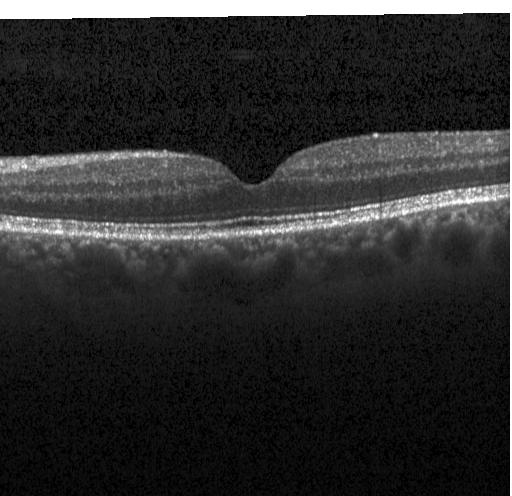
Assessment: no evidence of choroidal neovascularization, diabetic macular edema, or drusen.